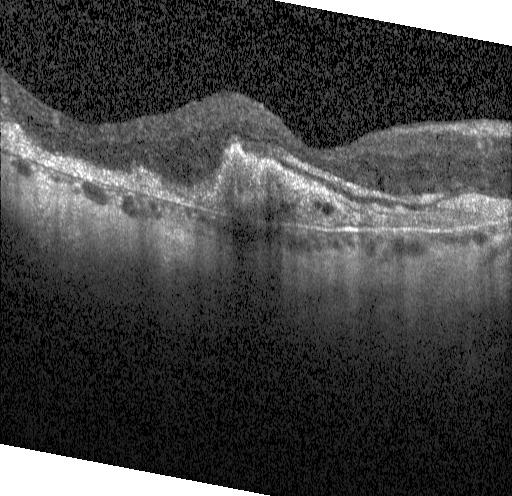
Spectral-domain OCT. Optical coherence tomography B-scan.
Impression: a choroidal neovascular membrane.